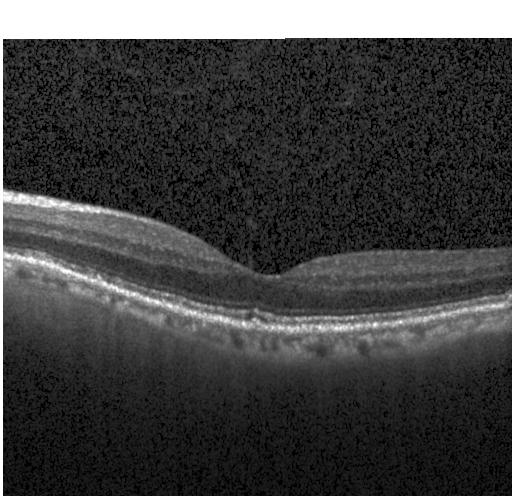

Retinal OCT cross-section. Fovea-centered. Diagnosis: neither choroidal neovascularization, diabetic macular edema, nor drusen.